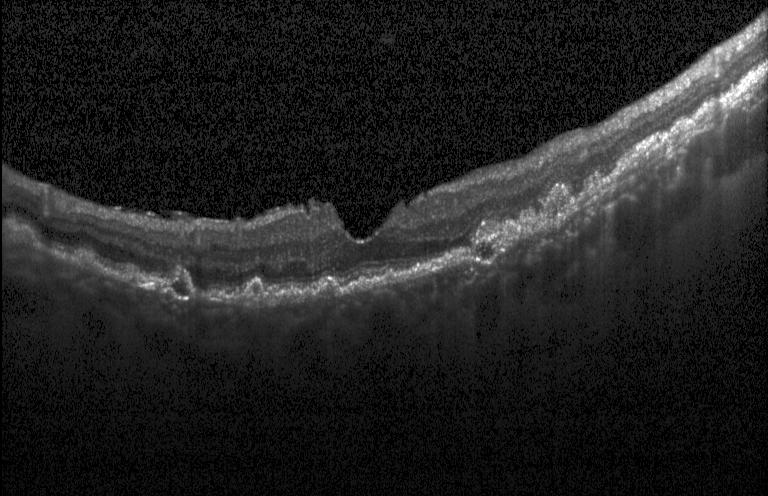 Heidelberg Spectralis OCT system · retinal OCT B-scan — This B-scan demonstrates CNV.